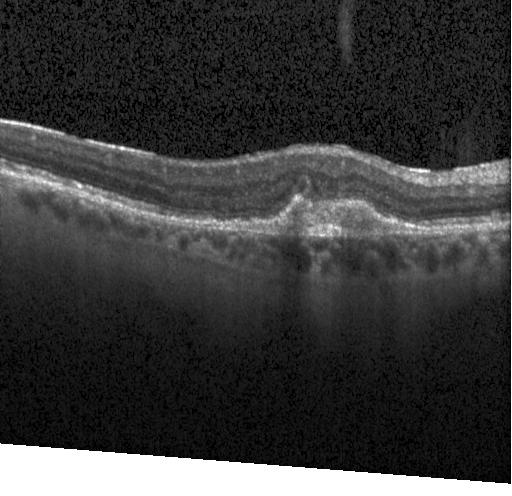 Spectral-domain OCT, Heidelberg Spectralis OCT system, OCT B-scan, centered on the fovea. Diagnosis: CNV.